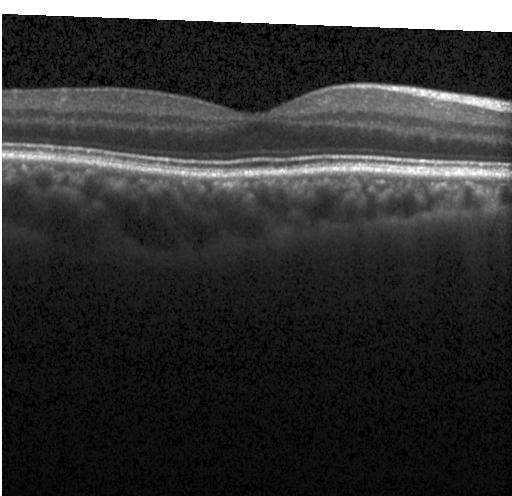 OCT finding: neither choroidal neovascularization, diabetic macular edema, nor drusen.